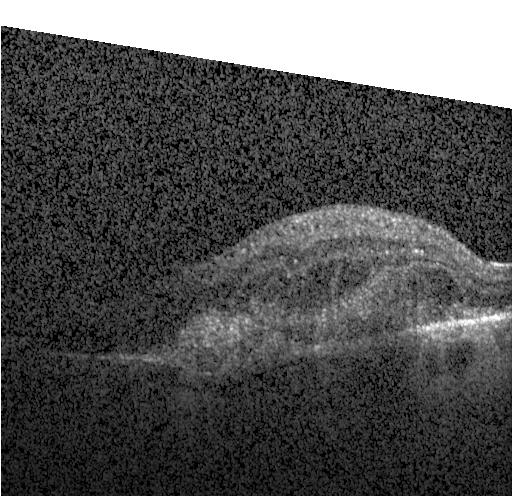
OCT B-scan
Dx: CNV.